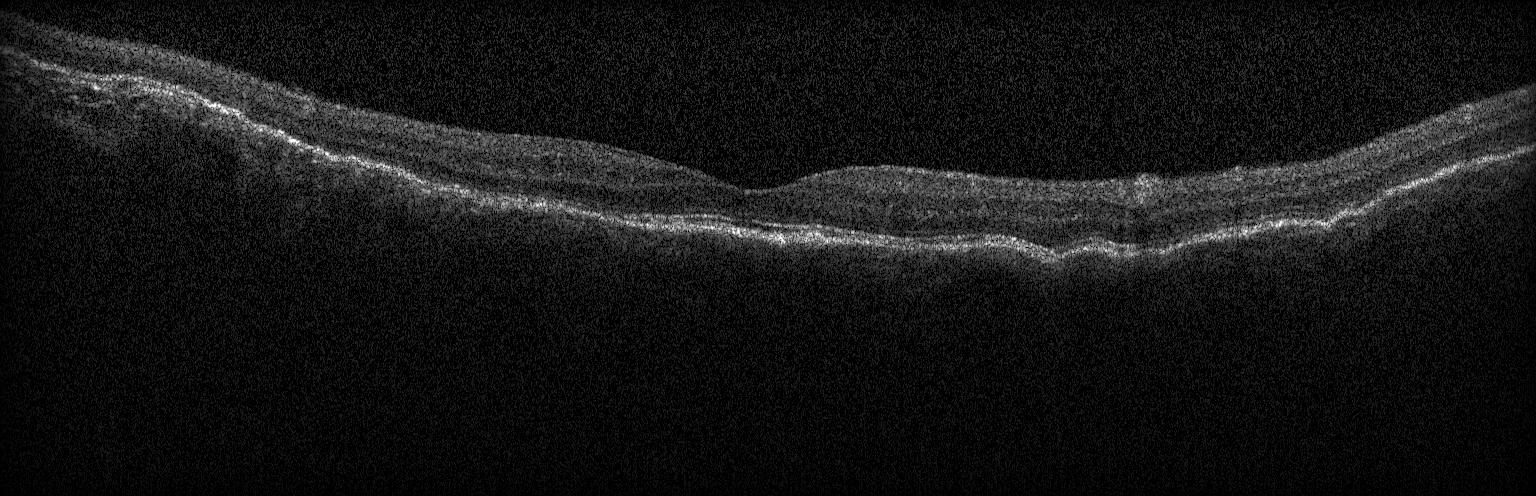 Finding: no CNV, no DME, and no drusen.